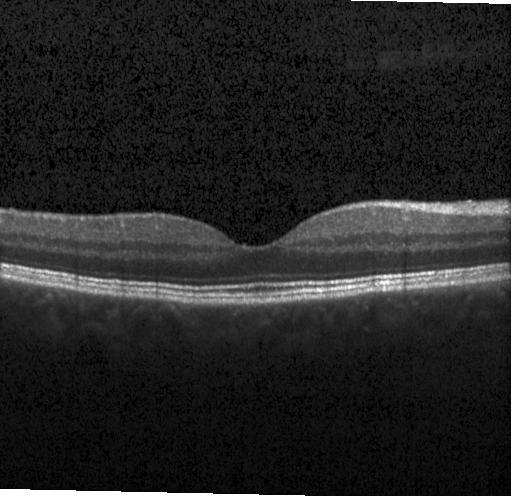
Optical coherence tomography B-scan. Centered on the fovea. SD-OCT. Acquired on a Heidelberg Spectralis.
Macular OCT: neither choroidal neovascularization, diabetic macular edema, nor drusen.